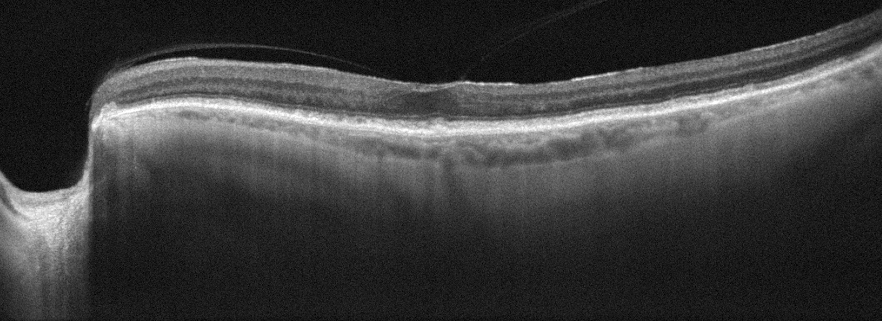
OS, retinal OCT B-scan — The scan shows epiretinal membrane.